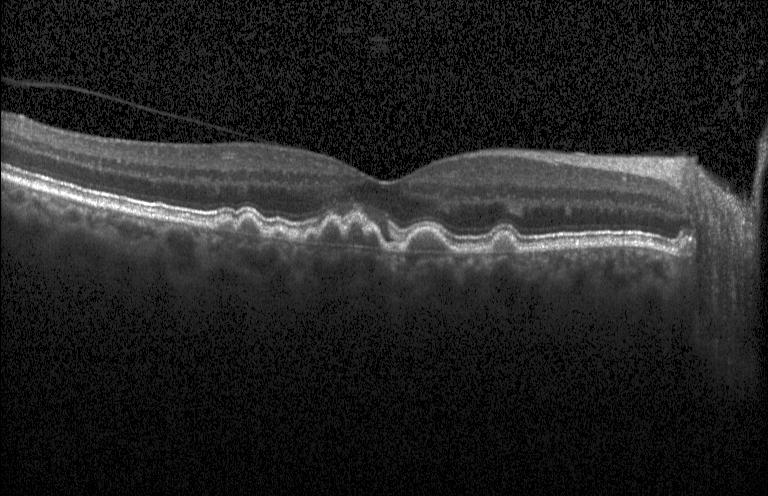
Macular OCT demonstrating multiple drusen.